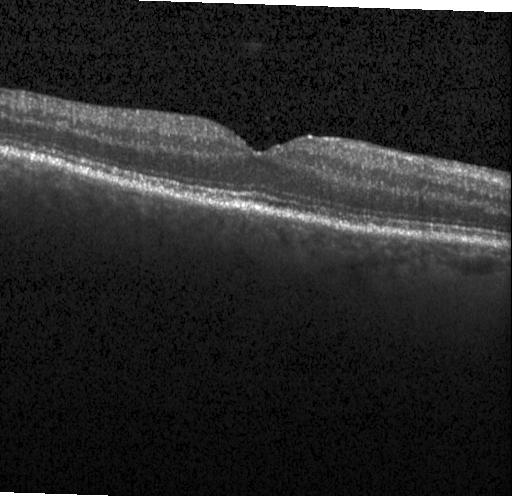
Optical coherence tomography scan; SD-OCT.
OCT finding: neither choroidal neovascularization, diabetic macular edema, nor drusen.